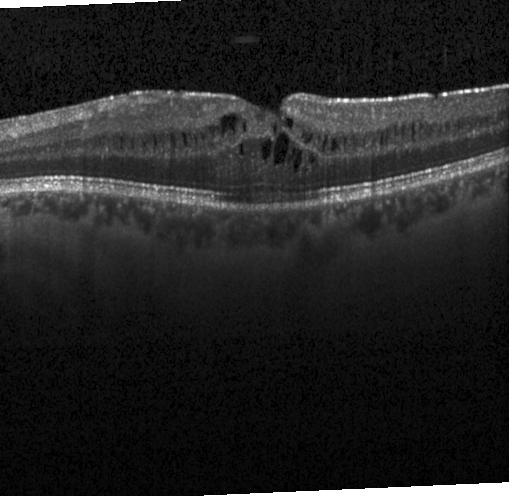
Acquired on a Heidelberg Spectralis, OCT B-scan
Assessment: DME.